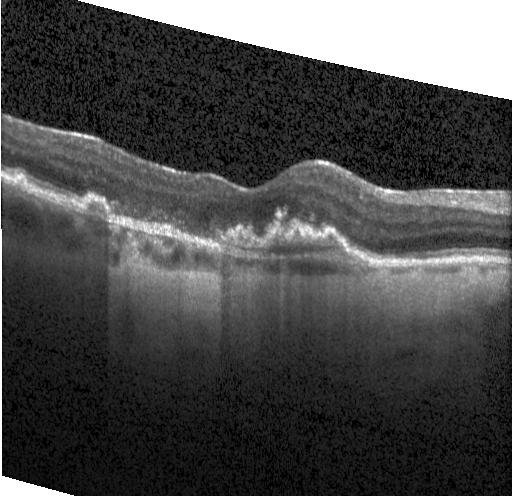 OCT B-scan. Macular OCT: choroidal neovascularization.